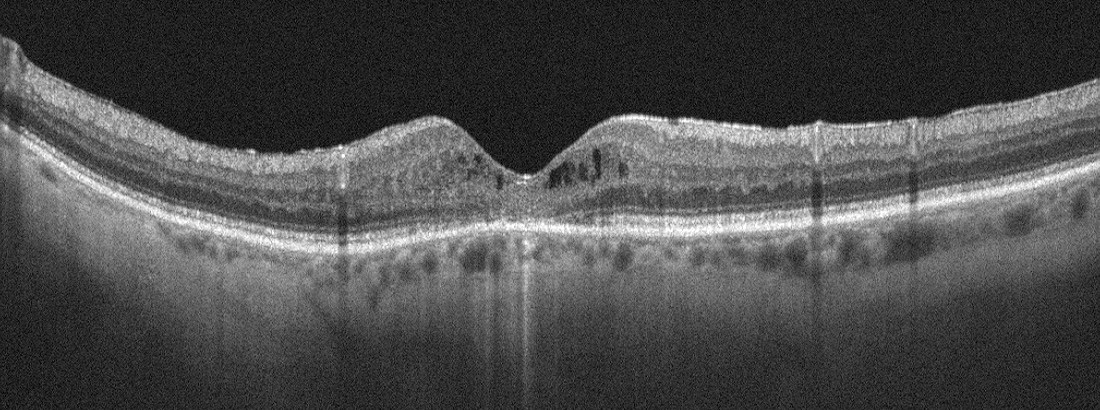

Instrument: Optovue Avanti RTVue XR · retinal OCT cross-section.
Impression: diabetic macular edema.